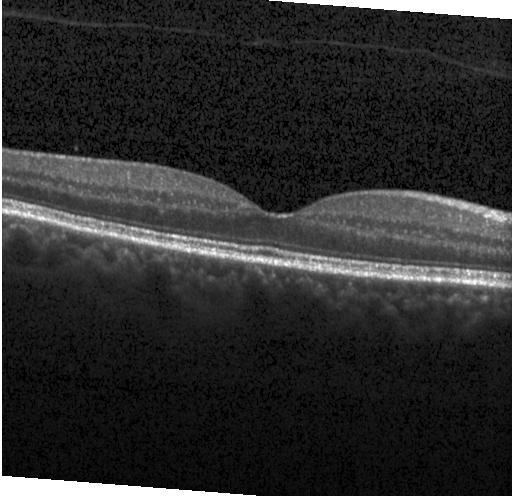
This B-scan demonstrates no choroidal neovascularization, diabetic macular edema, or drusen.